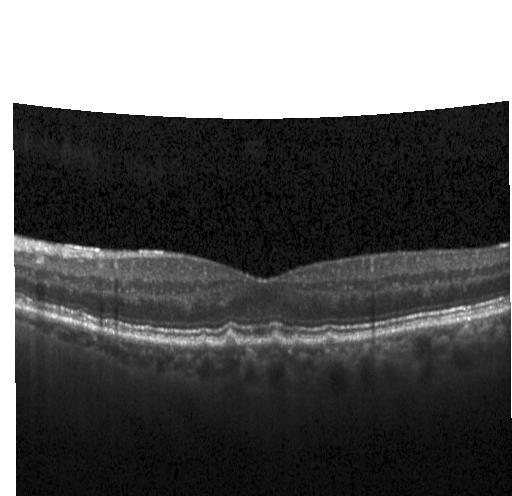
Diagnosis: multiple drusen.